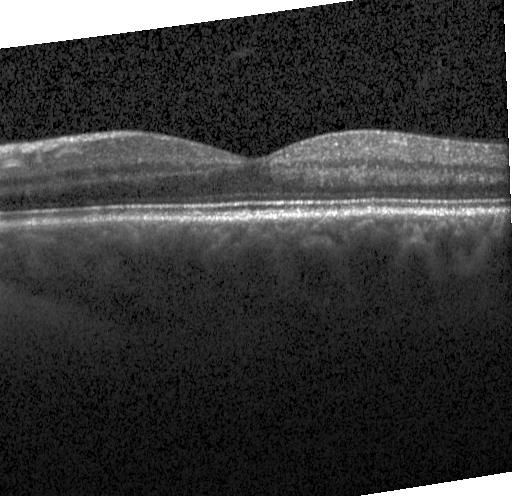
OCT scan showing no evidence of CNV, DME, or drusen.